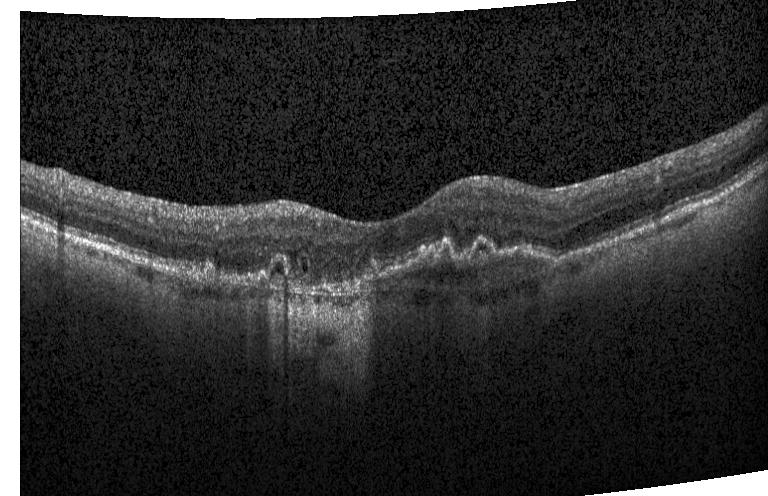 This B-scan demonstrates choroidal neovascularization (CNV).